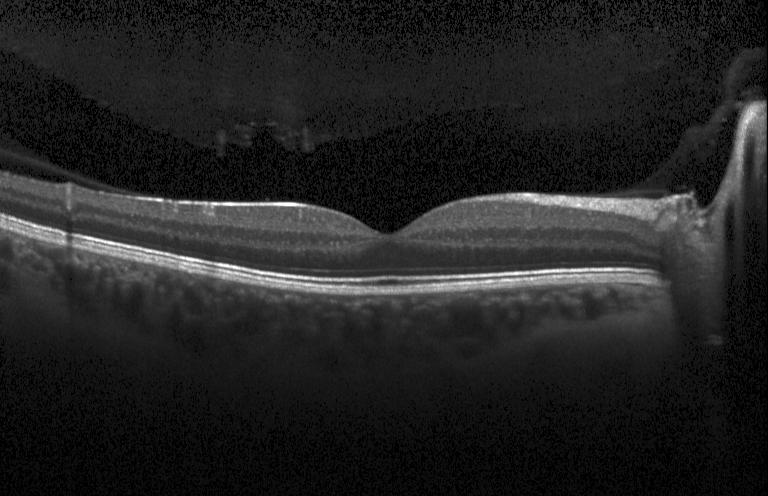 Optical coherence tomography B-scan — Assessment: neither choroidal neovascularization, diabetic macular edema, nor drusen.